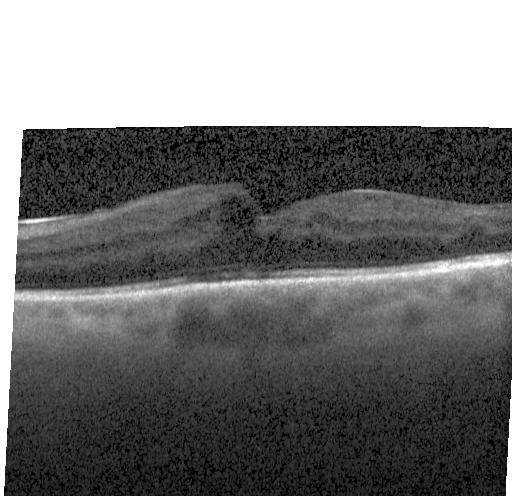 Optical coherence tomography scan · Heidelberg Spectralis — OCT finding: diabetic macular edema.